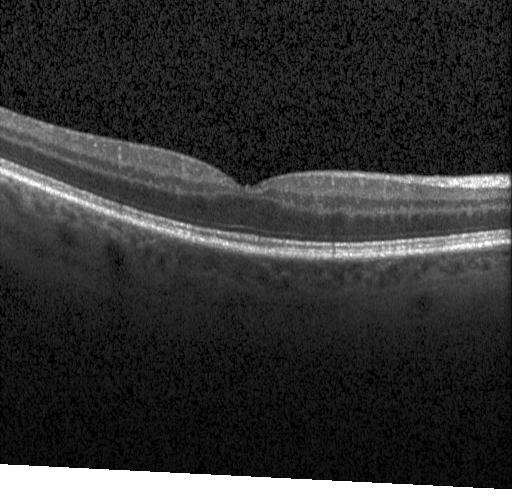 This B-scan demonstrates no choroidal neovascularization, no diabetic macular edema, and no drusen.